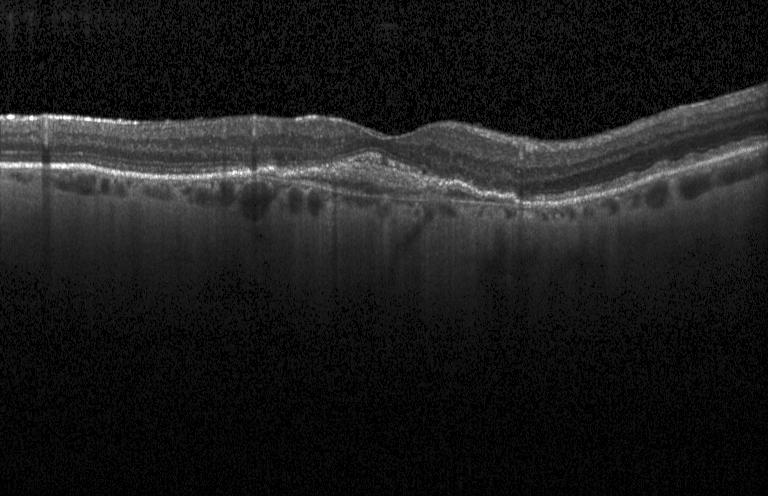 This B-scan demonstrates a choroidal neovascular membrane.